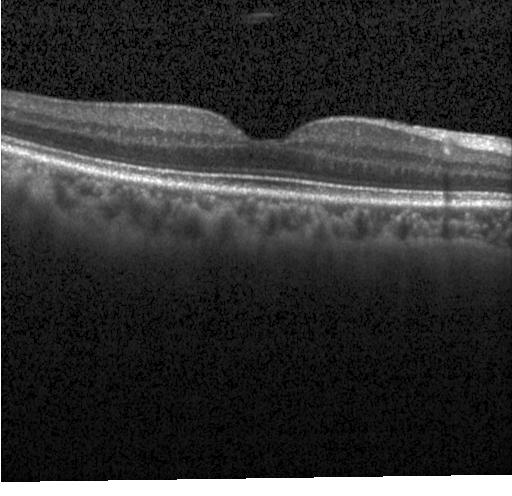 OCT B-scan — Finding: no CNV, no DME, and no drusen.